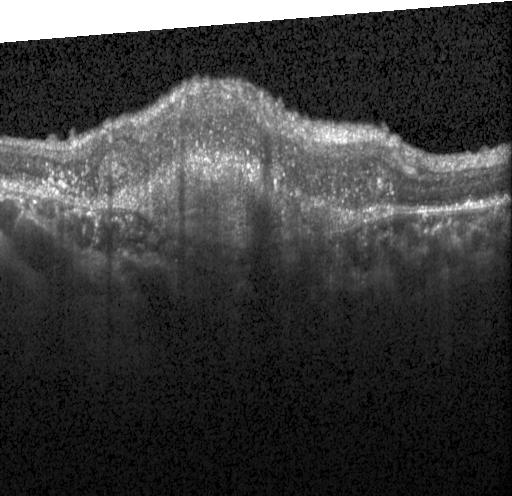
Impression: a choroidal neovascular membrane.